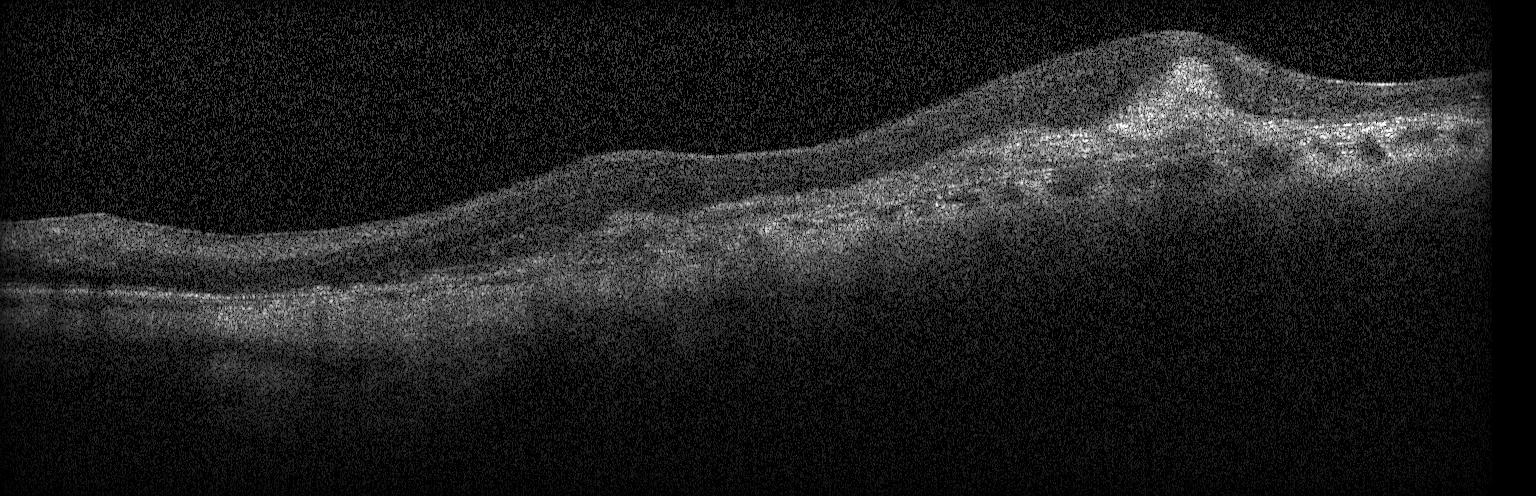 Instrument: Heidelberg Spectralis, macular scan, optical coherence tomography scan. Impression: a choroidal neovascular membrane.